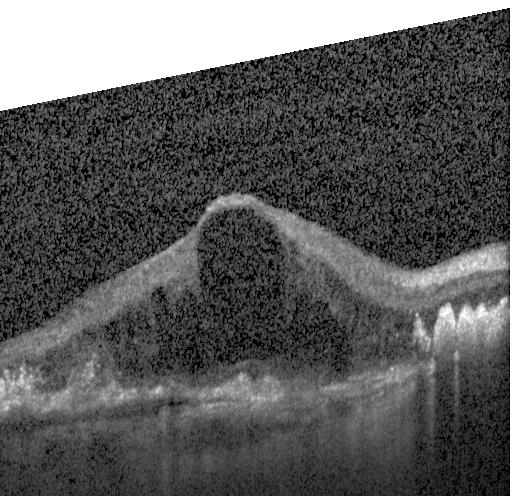

Impression: a choroidal neovascular membrane.